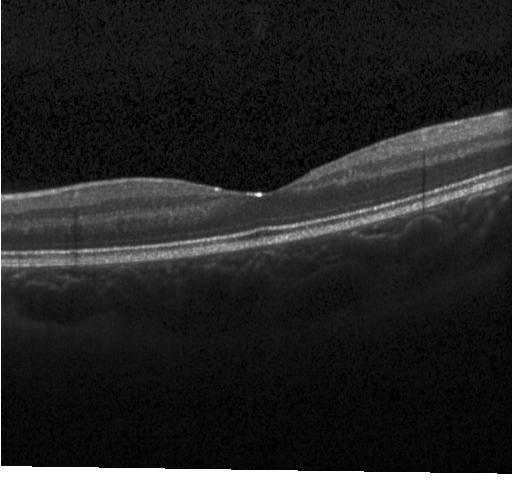

Fovea-centered · retinal OCT cross-section — Finding: no CNV, DME, or drusen.